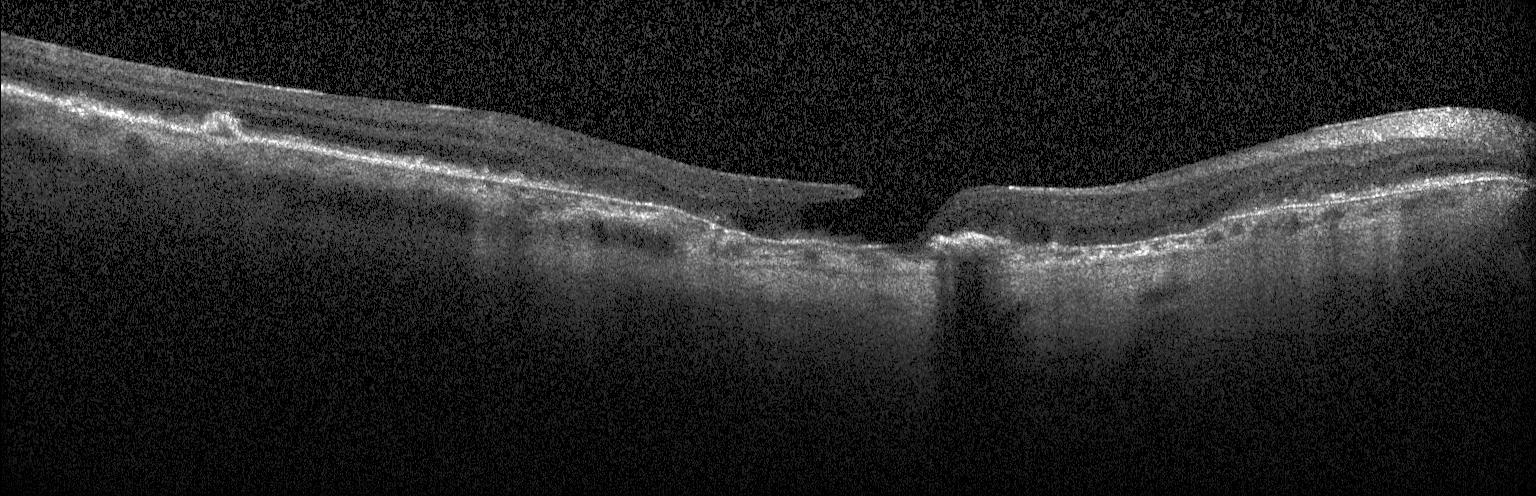 This B-scan demonstrates a choroidal neovascular membrane.